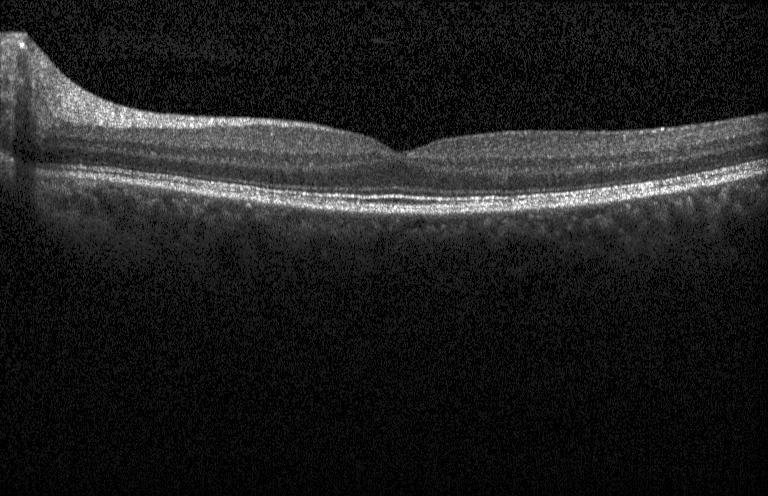

Spectral-domain optical coherence tomography, optical coherence tomography scan
No choroidal neovascularization, diabetic macular edema, or drusen.